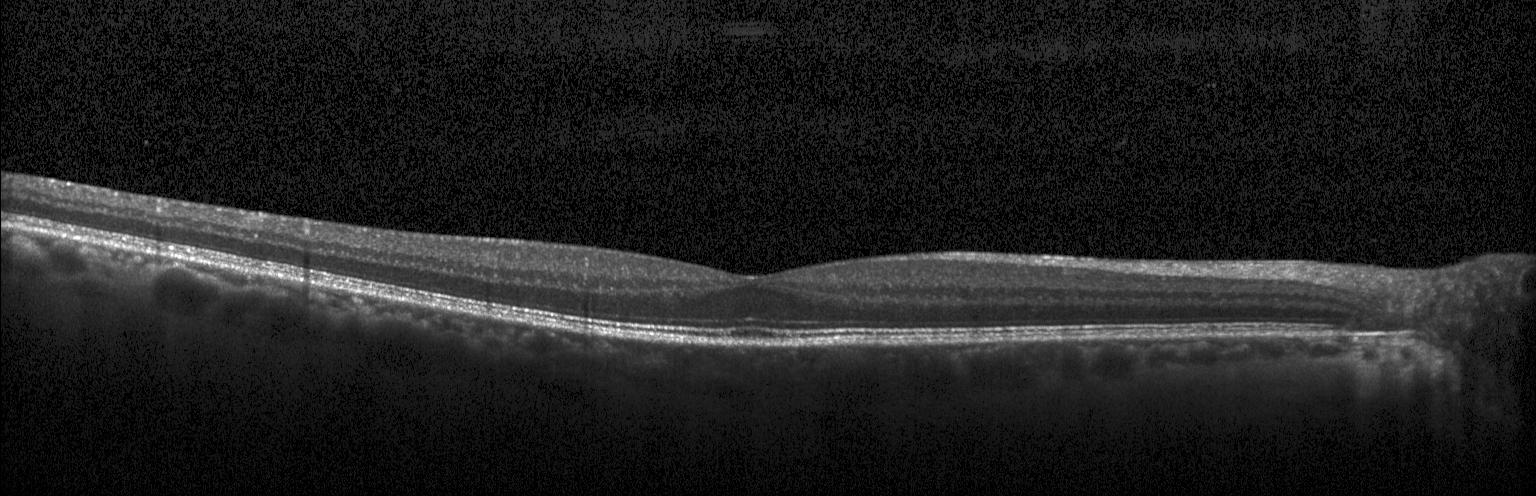

Heidelberg Spectralis OCT system · OCT line scan.
Impression: no choroidal neovascularization, no diabetic macular edema, and no drusen.